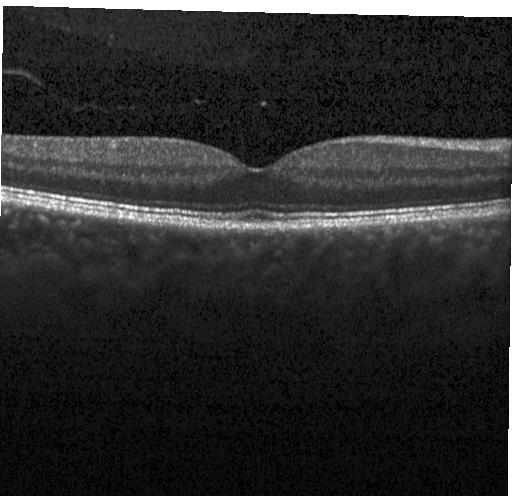

Centered on the fovea. Spectral-domain OCT. Optical coherence tomography scan. Heidelberg Spectralis OCT system
OCT finding: no CNV, DME, or drusen.